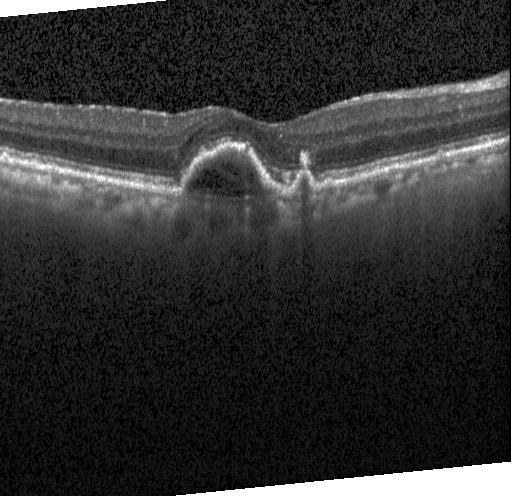

OCT B-scan. Instrument: Heidelberg Spectralis. Macular scan.
Dx: a choroidal neovascular membrane.